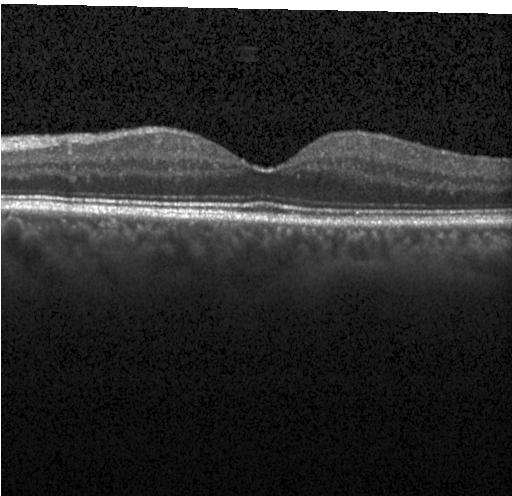
Optical coherence tomography scan.
Finding: no evidence of CNV, DME, or drusen.